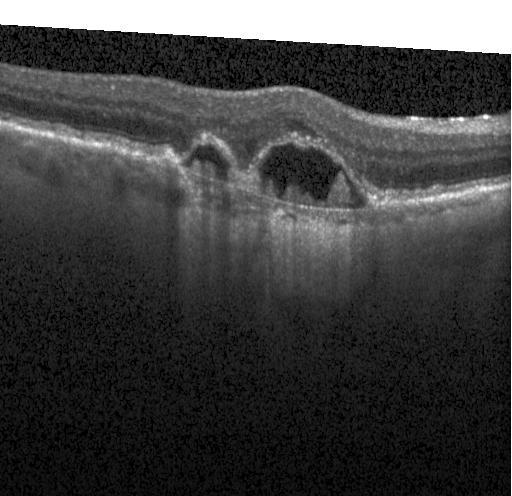

Spectral-domain OCT · centered on the fovea · retinal OCT B-scan.
Impression: choroidal neovascularization (CNV).